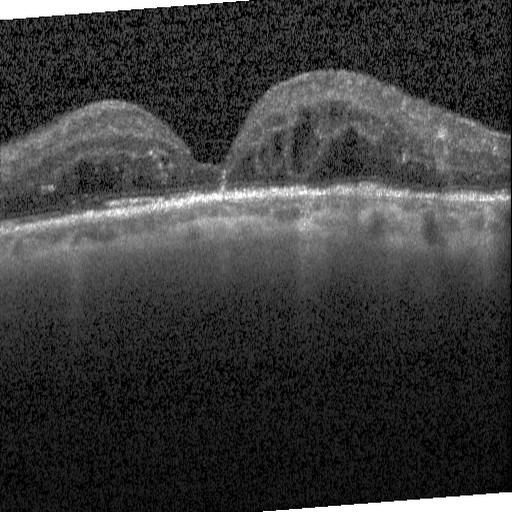
OCT line scan.
OCT finding: DME.